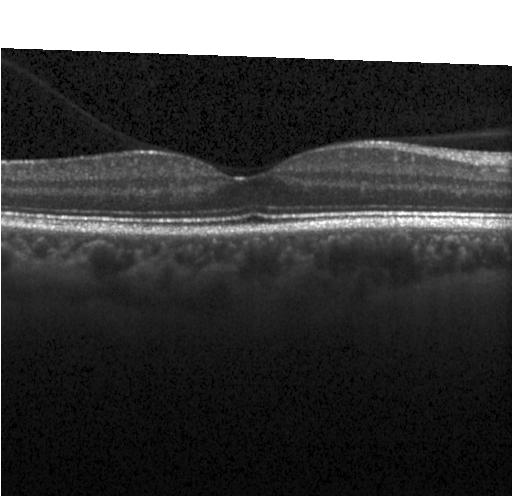
Through the macula; acquired on a Heidelberg Spectralis; spectral-domain optical coherence tomography; optical coherence tomography scan
OCT finding: no CNV, no DME, and no drusen.